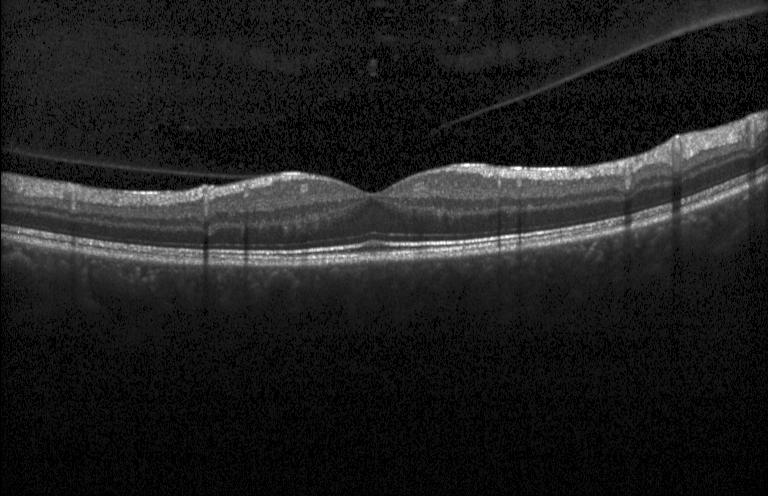
SD-OCT · optical coherence tomography scan · Heidelberg Spectralis OCT system.
Impression: neither choroidal neovascularization, diabetic macular edema, nor drusen.